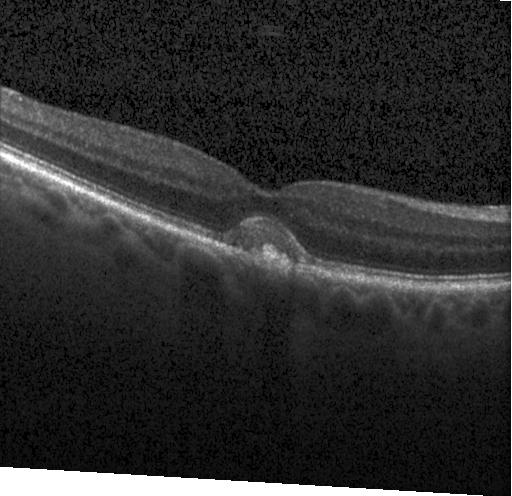 Instrument: Heidelberg Spectralis; through the macula; retinal OCT B-scan
Impression: a choroidal neovascular membrane.